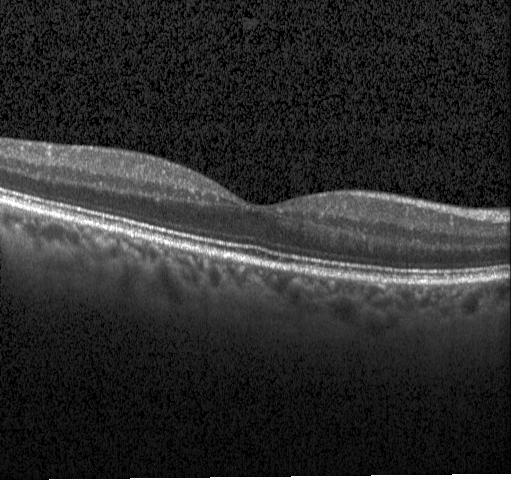 Through the macula · spectral-domain optical coherence tomography · optical coherence tomography scan — Dx: neither CNV, DME, nor drusen.